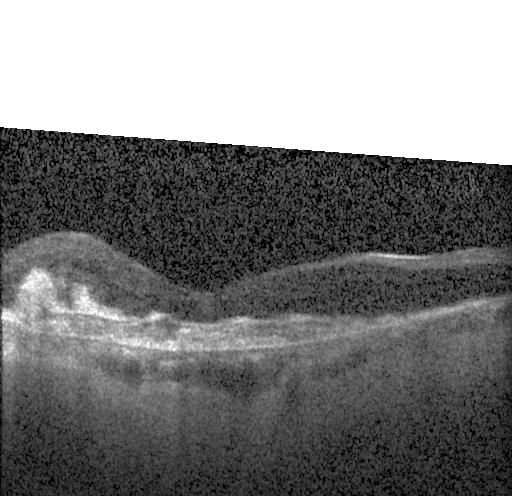 Instrument: Heidelberg Spectralis, SD-OCT, optical coherence tomography scan, through the macula
Diagnosis: a choroidal neovascular membrane.